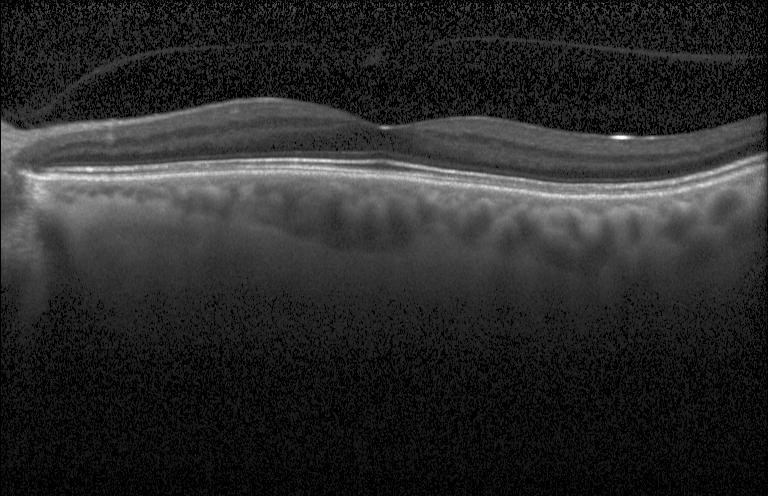

Retinal OCT B-scan. OCT finding: neither choroidal neovascularization, diabetic macular edema, nor drusen.